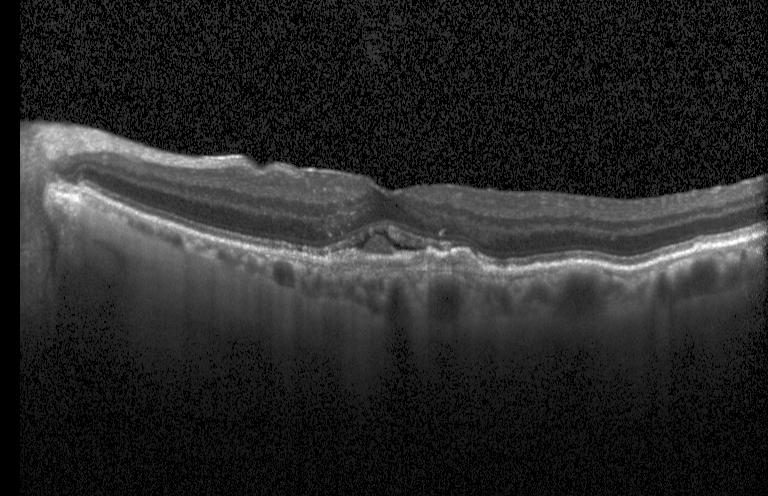 Macular OCT: CNV.